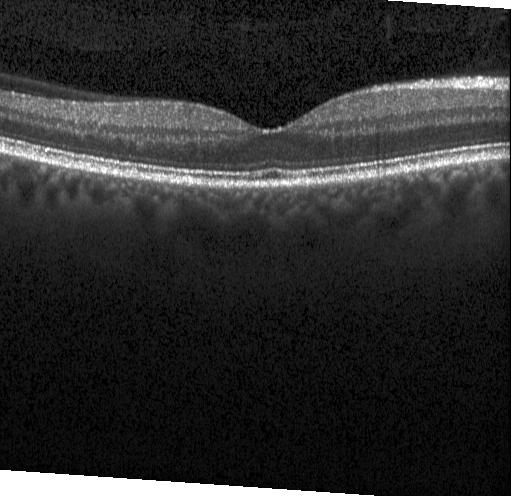
Spectral-domain OCT; macular scan; OCT B-scan — Impression: no choroidal neovascularization, no diabetic macular edema, and no drusen.